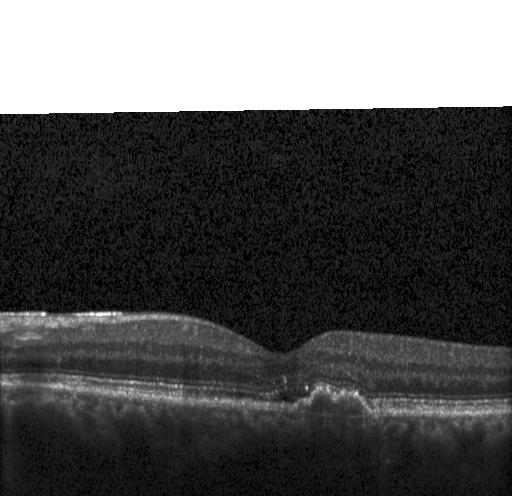

Optical coherence tomography scan — Diagnosis: CNV.